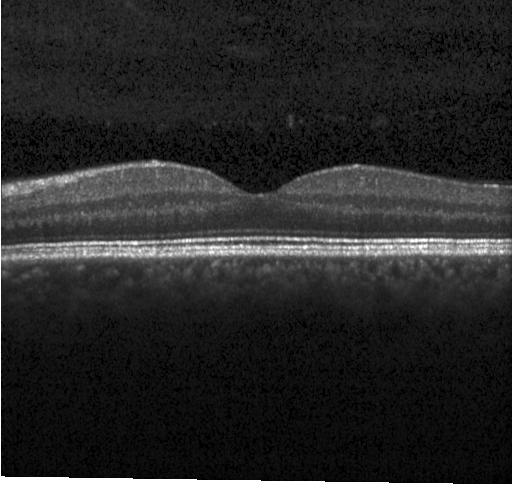
Retinal OCT B-scan
This B-scan demonstrates no CNV, DME, or drusen.